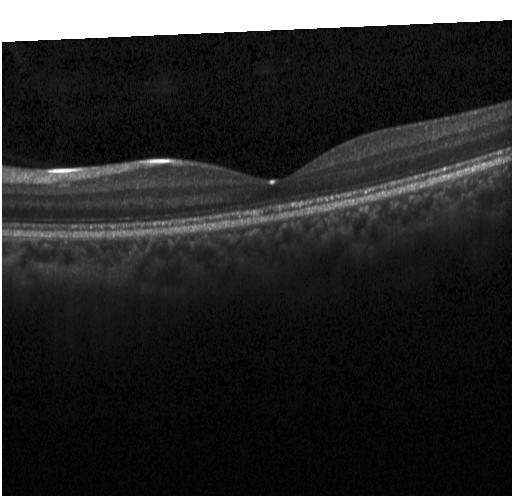 OCT B-scan
Impression: no choroidal neovascularization, diabetic macular edema, or drusen.